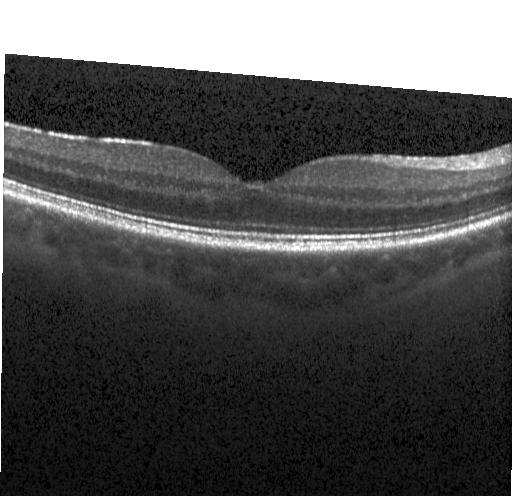 Retinal OCT B-scan, macular scan. Diagnosis: no choroidal neovascularization, no diabetic macular edema, and no drusen.